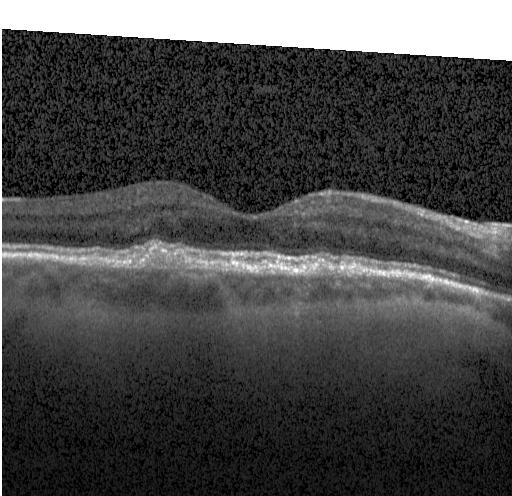
Impression: multiple drusen.